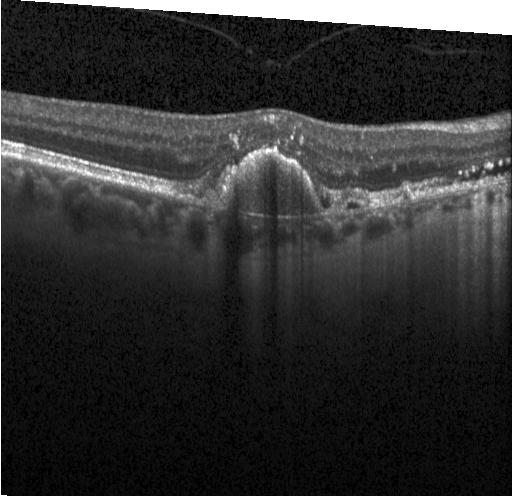

Optical coherence tomography scan.
Diagnosis: a choroidal neovascular membrane.